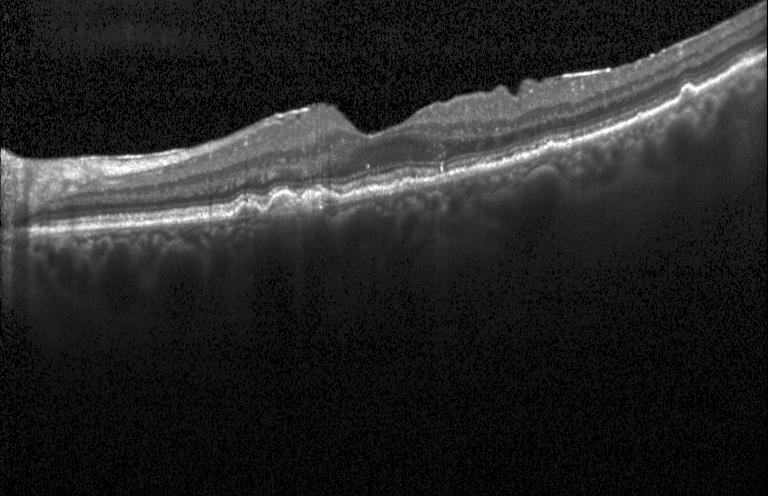 OCT finding: multiple drusen.